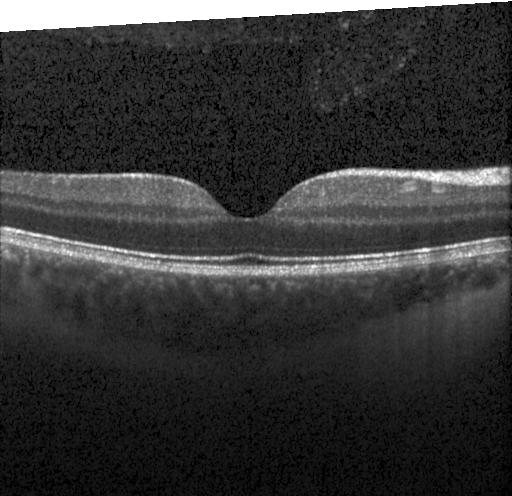 OCT line scan, fovea-centered.
Finding: no CNV, DME, or drusen.